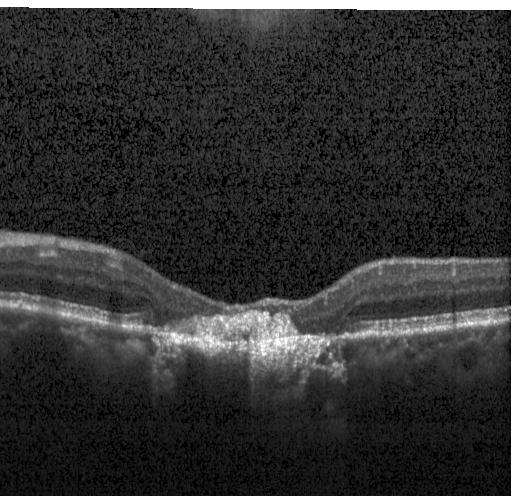
OCT B-scan.
Impression: a choroidal neovascular membrane.